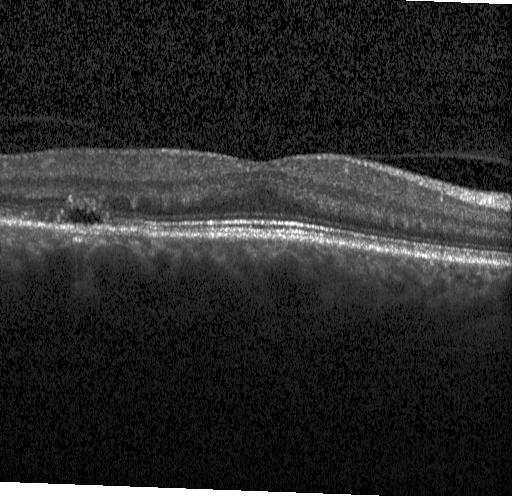
Horizontal scan through the fovea · SD-OCT · OCT line scan — Diagnosis: a choroidal neovascular membrane.